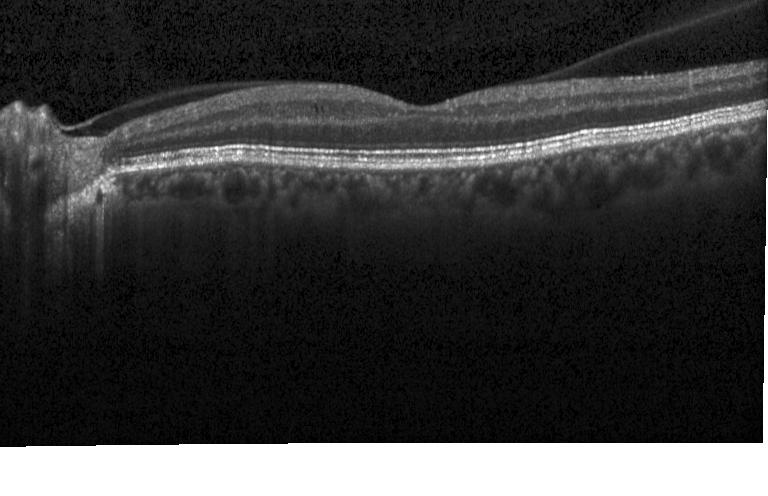
Macular OCT: no CNV, DME, or drusen.